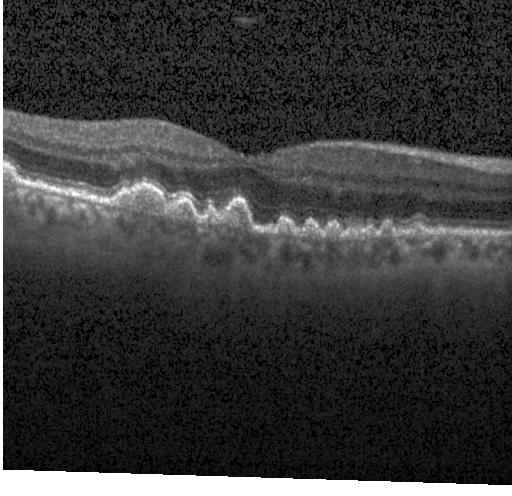

Spectral-domain optical coherence tomography. OCT line scan — Macular OCT: drusen.